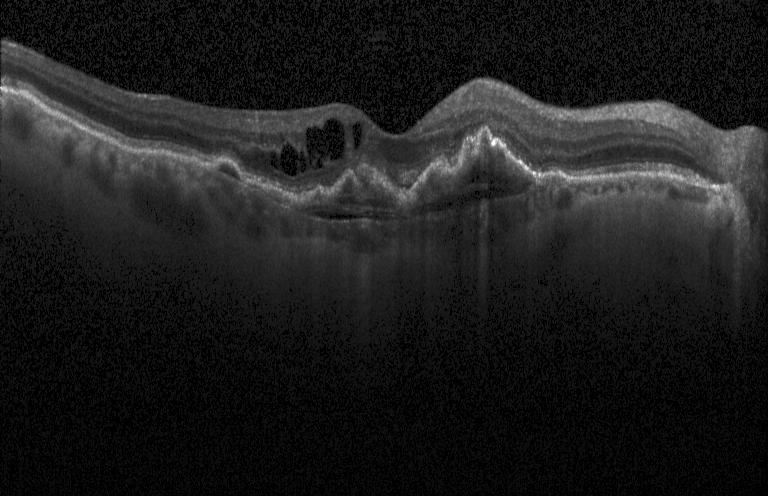

Spectral-domain OCT; retinal OCT B-scan; centered on the fovea
Finding: a choroidal neovascular membrane.